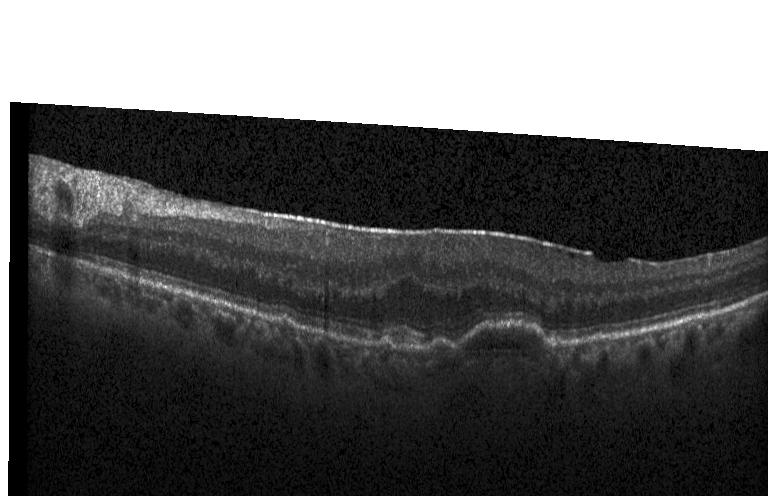
Spectral-domain OCT · horizontal scan through the fovea · OCT line scan.
Finding: choroidal neovascularization (CNV).